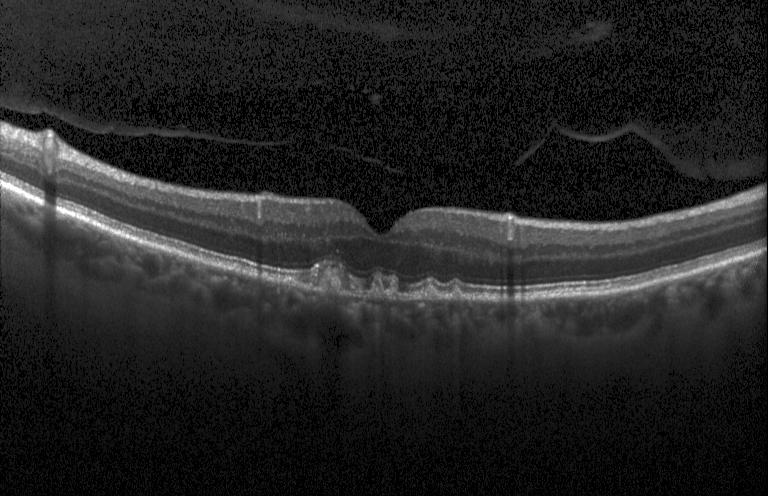 Macular OCT: drusen.